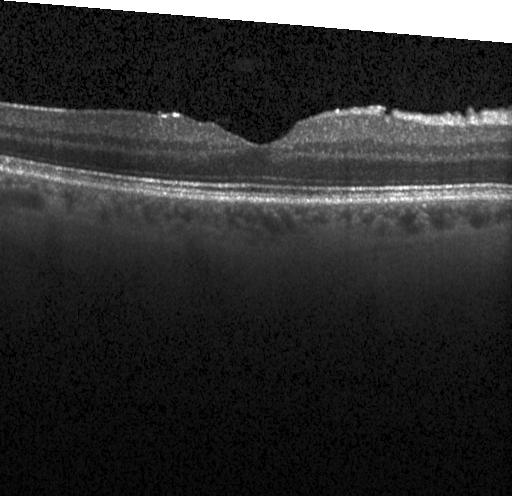

Finding: no evidence of choroidal neovascularization, diabetic macular edema, or drusen.